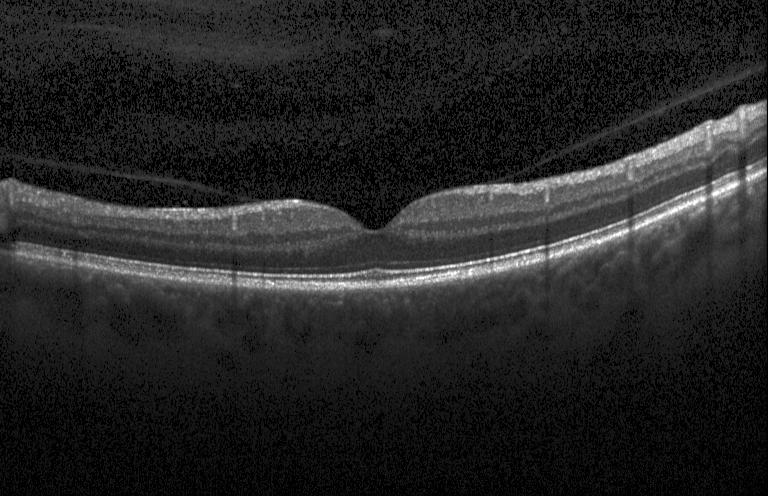 Retinal OCT cross-section — Impression: neither choroidal neovascularization, diabetic macular edema, nor drusen.